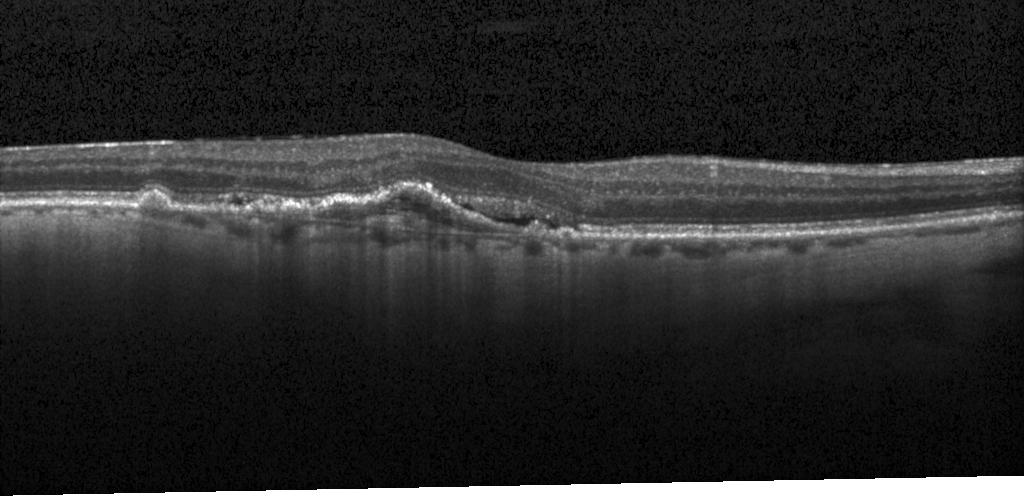 Macular scan · spectral-domain OCT · retinal OCT B-scan · instrument: Heidelberg Spectralis
OCT finding: a choroidal neovascular membrane.